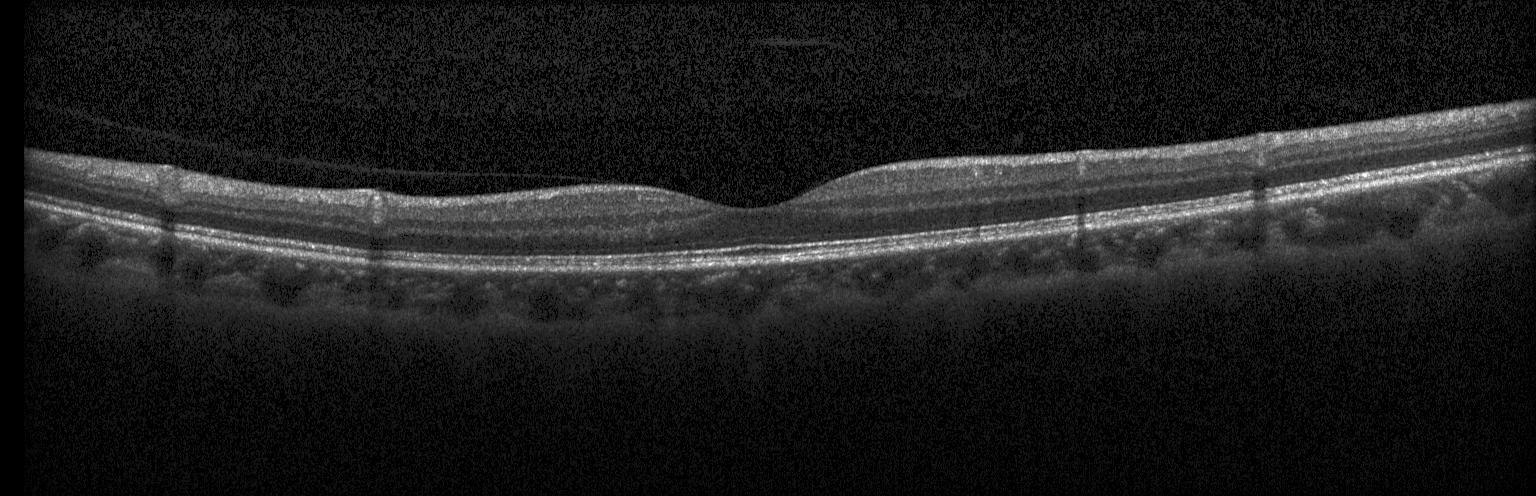
Optical coherence tomography B-scan · SD-OCT · through the macula · instrument: Heidelberg Spectralis. No evidence of CNV, DME, or drusen.